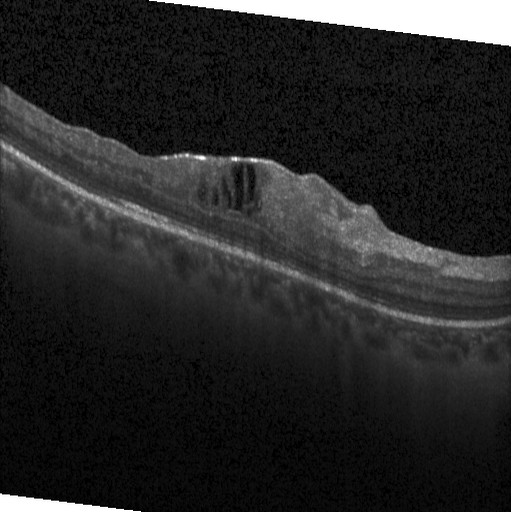 OCT line scan. Assessment: diabetic macular edema (DME).